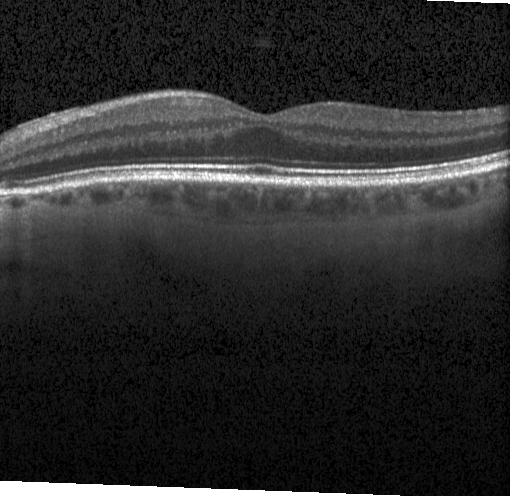
Finding: no CNV, no DME, and no drusen.